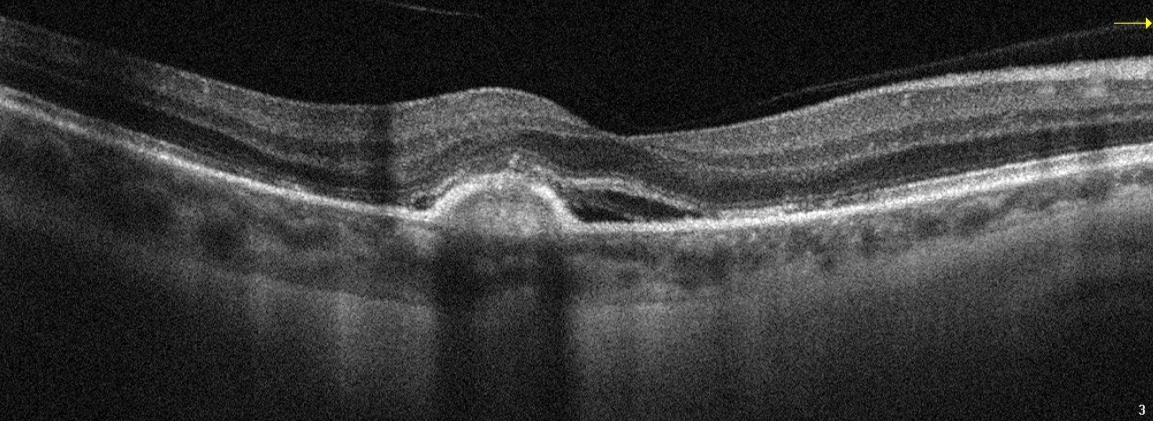 Macular scan · instrument: Optovue Avanti RTVue XR · OCT B-scan — Finding: age-related macular degeneration.